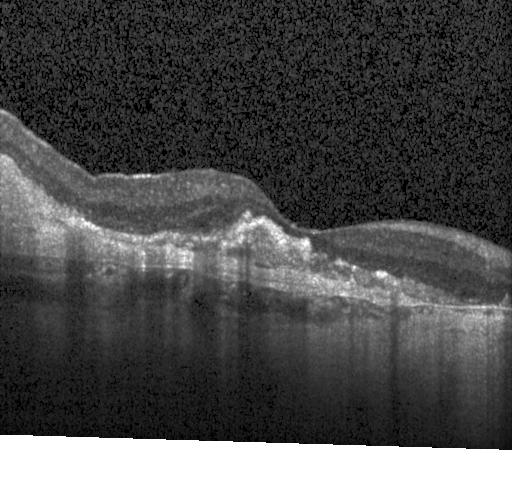

OCT line scan
Finding: a choroidal neovascular membrane.